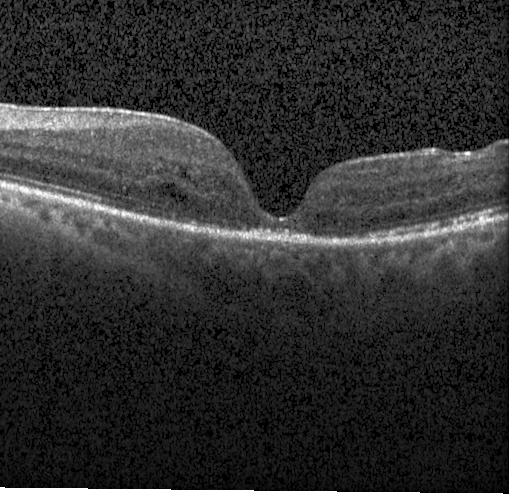

SD-OCT. Optical coherence tomography B-scan
Diabetic macular edema.